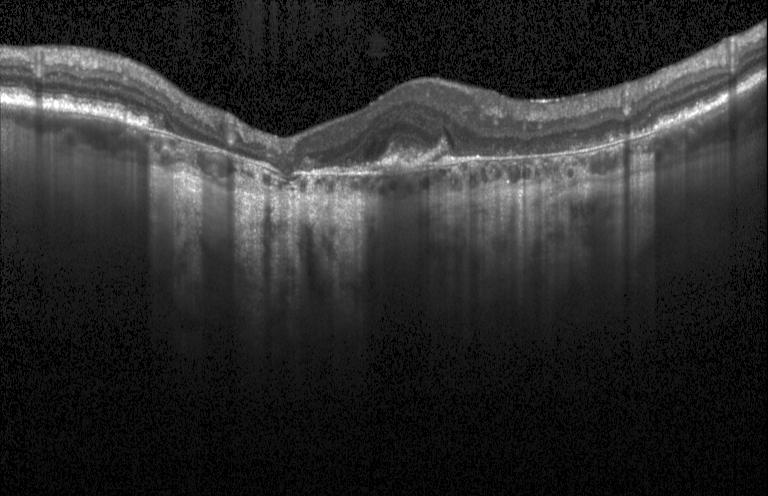 Diagnosis: a choroidal neovascular membrane.